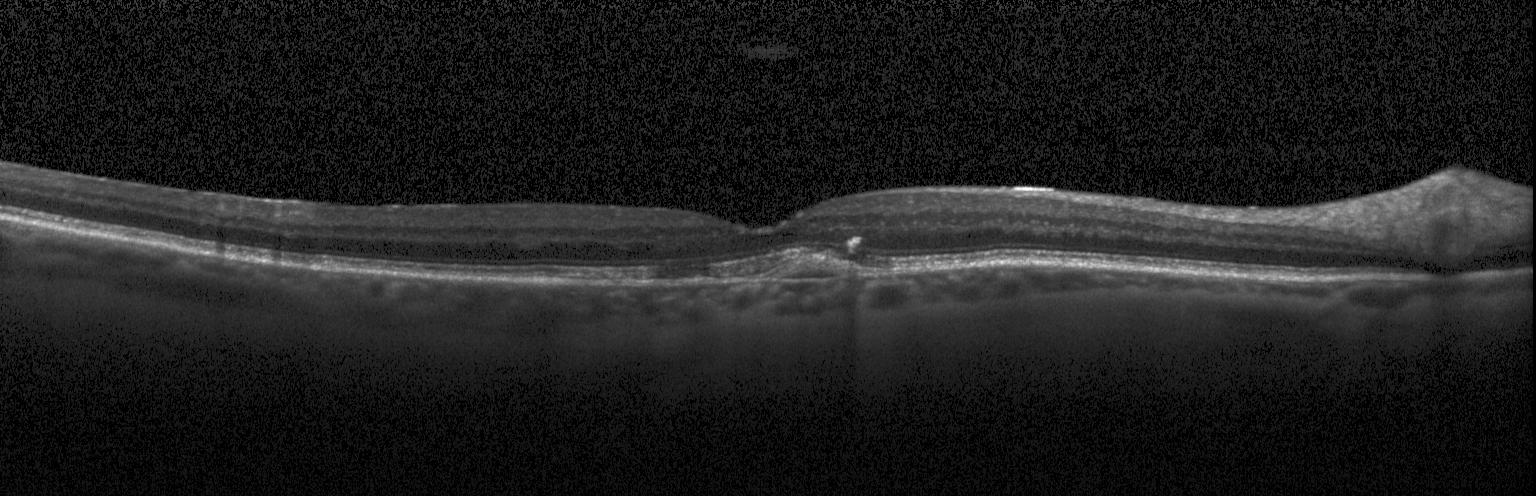
Retinal OCT B-scan. Instrument: Heidelberg Spectralis. Finding: CNV.